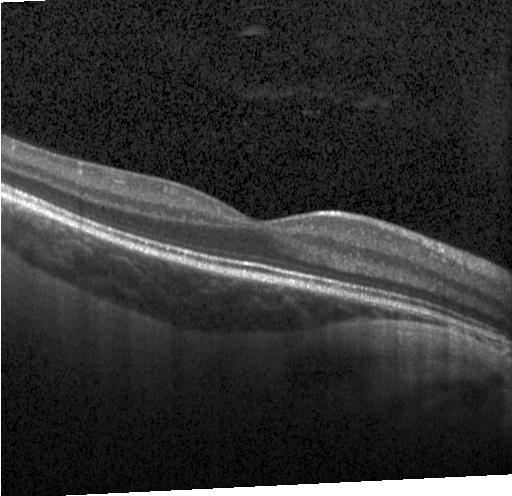 OCT line scan.
Finding: no evidence of CNV, DME, or drusen.